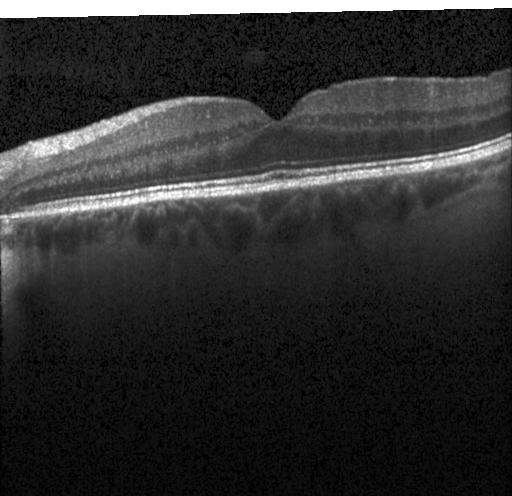

Optical coherence tomography scan. Fovea-centered. Heidelberg Spectralis. Impression: no CNV, DME, or drusen.